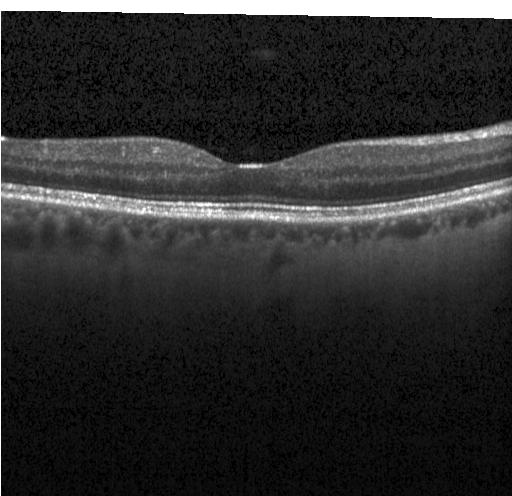

Retinal OCT cross-section · acquired on a Heidelberg Spectralis
Diagnosis: no CNV, no DME, and no drusen.